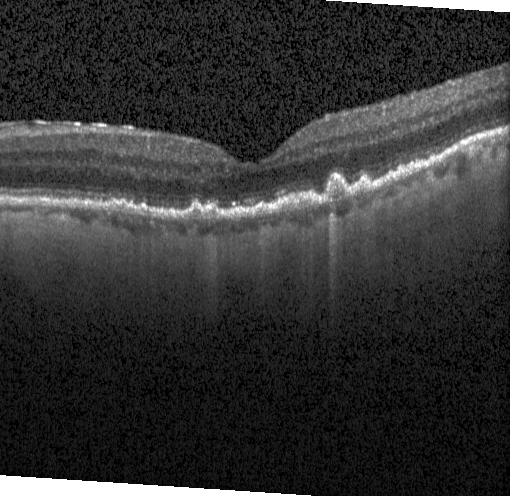 SD-OCT; Heidelberg Spectralis; optical coherence tomography scan. Sub-RPE drusenoid deposits.